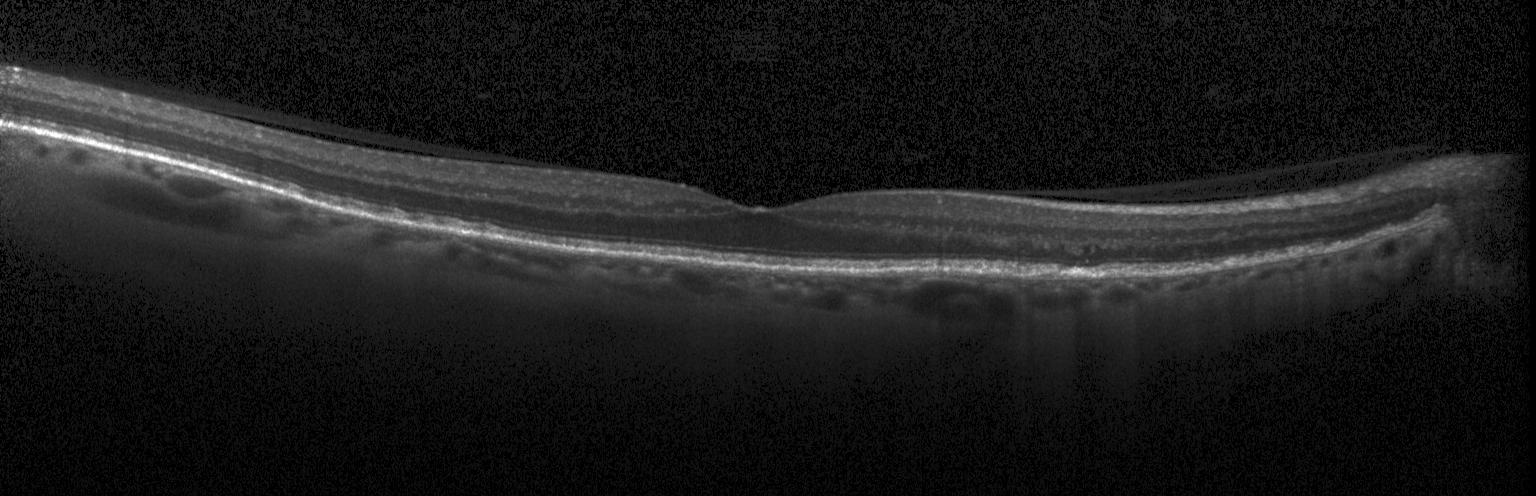
Macular OCT demonstrating no choroidal neovascularization, diabetic macular edema, or drusen.